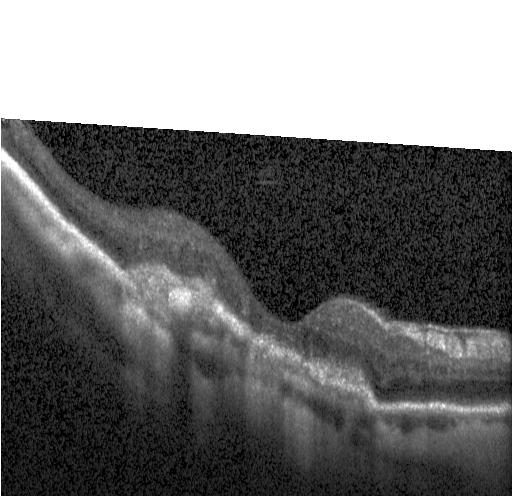
Horizontal scan through the fovea · optical coherence tomography B-scan.
CNV.